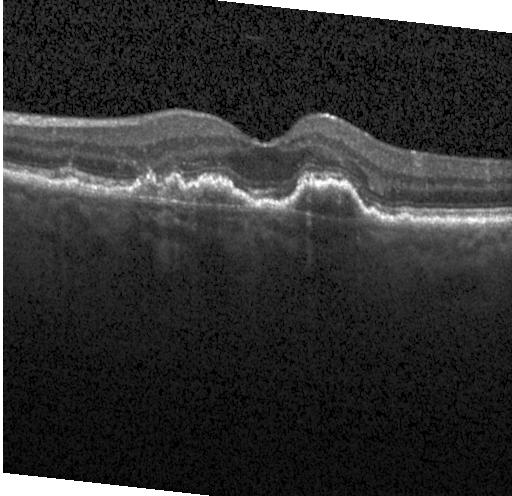
OCT B-scan. Centered on the fovea. Spectral-domain OCT. Assessment: a choroidal neovascular membrane.